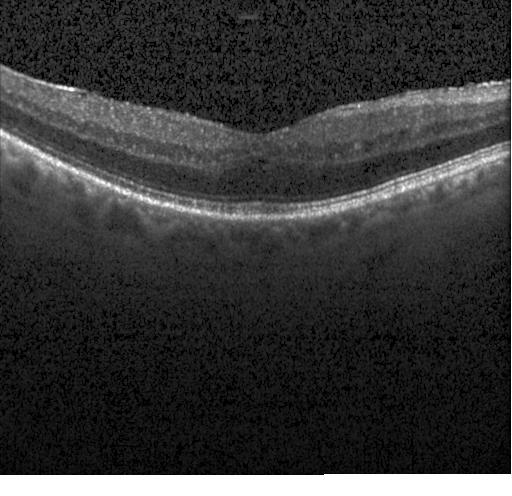
Finding: no evidence of CNV, DME, or drusen.